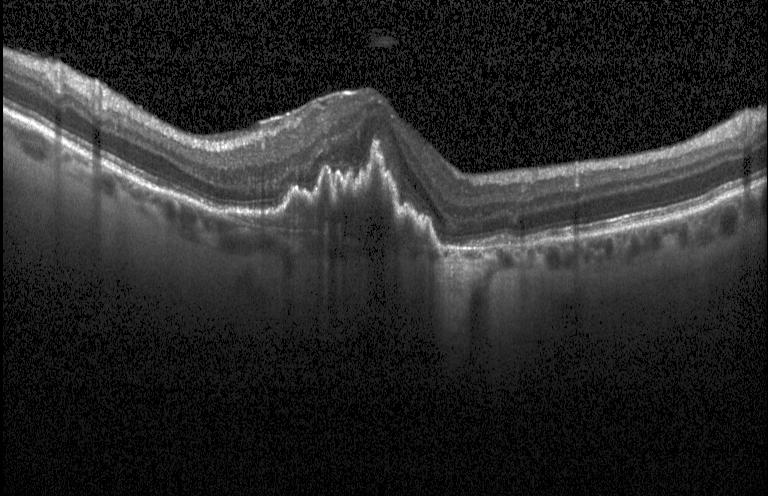
Heidelberg Spectralis OCT system, centered on the fovea, optical coherence tomography B-scan — Impression: a choroidal neovascular membrane.